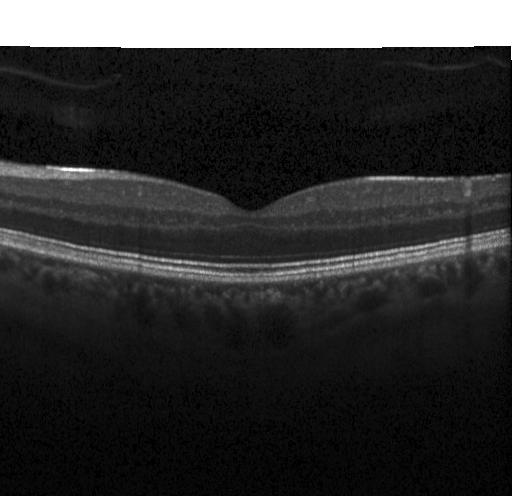

Retinal OCT cross-section — Macular OCT: no CNV, no DME, and no drusen.